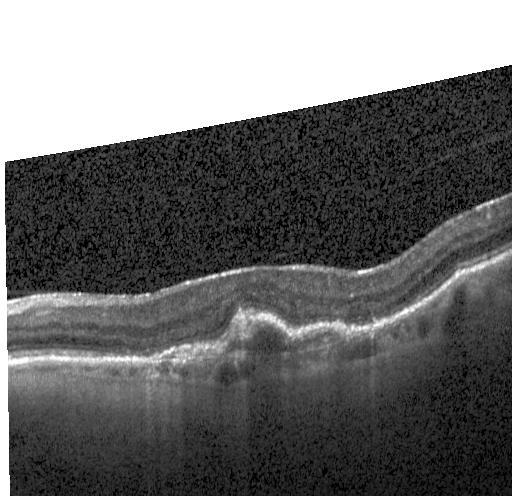 OCT line scan; Heidelberg Spectralis OCT system; centered on the fovea. Impression: a choroidal neovascular membrane.